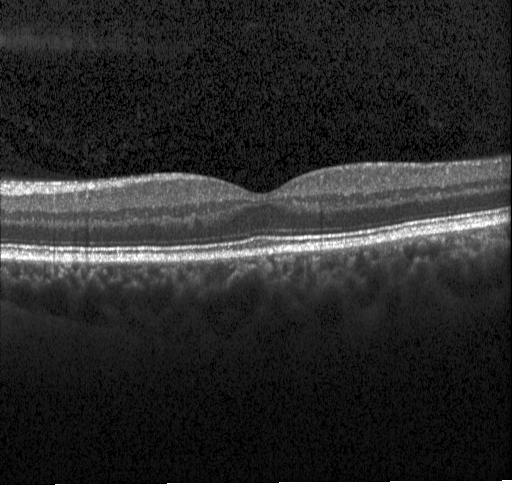

OCT finding: neither choroidal neovascularization, diabetic macular edema, nor drusen.